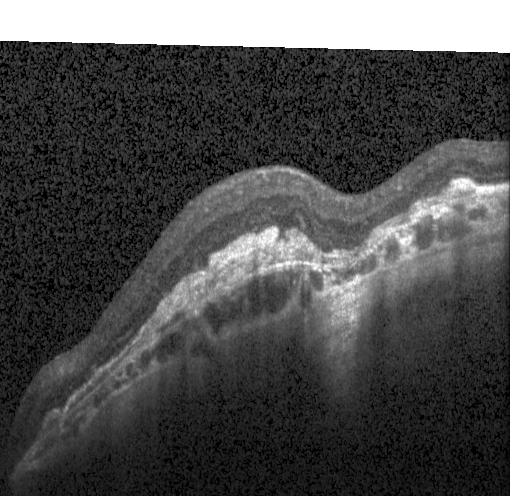

Optical coherence tomography scan. The scan shows choroidal neovascularization.